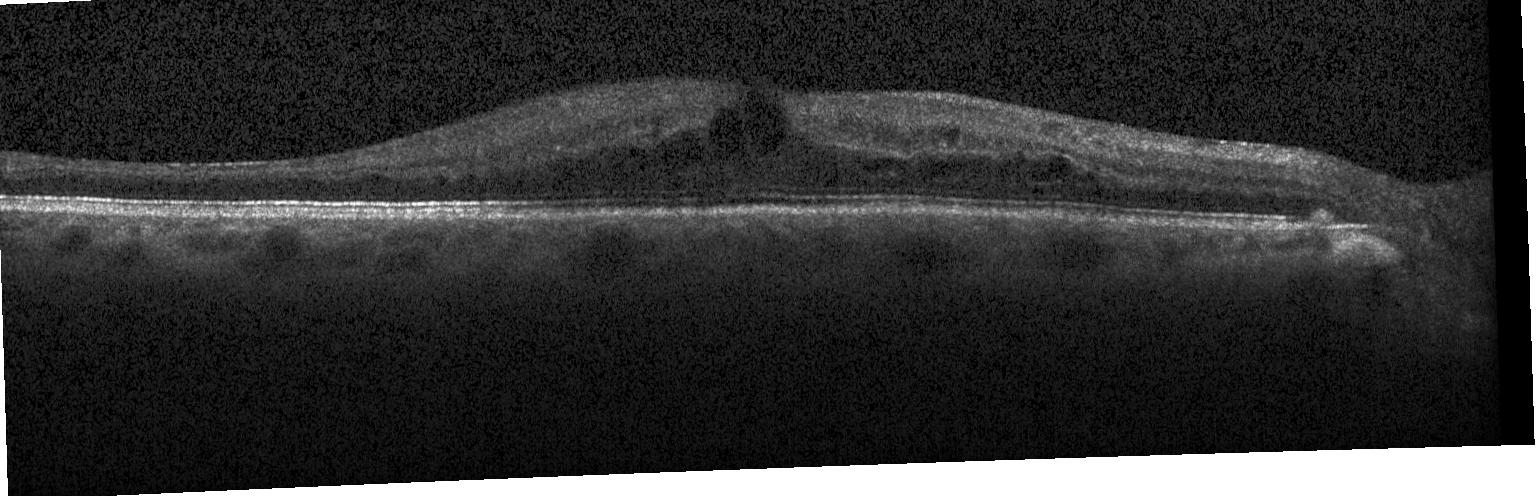
Retinal OCT B-scan · Heidelberg Spectralis · horizontal scan through the fovea · spectral-domain OCT — Macular OCT: diabetic macular edema.